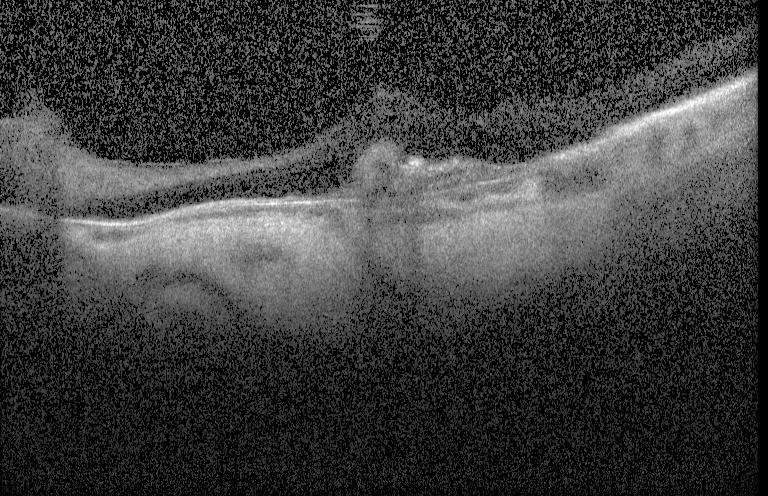 Dx: CNV.